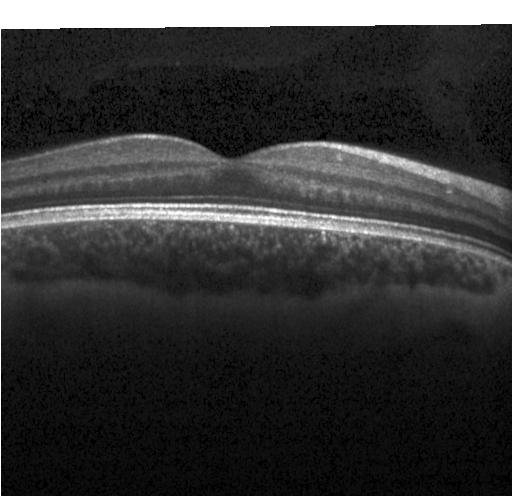
Finding: no choroidal neovascularization, no diabetic macular edema, and no drusen.